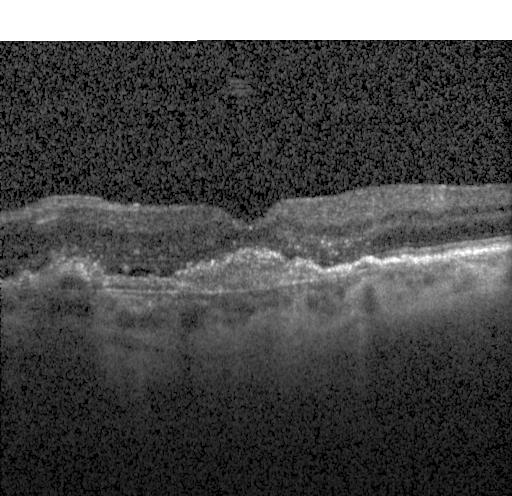 Spectral-domain optical coherence tomography; retinal OCT cross-section — A choroidal neovascular membrane.